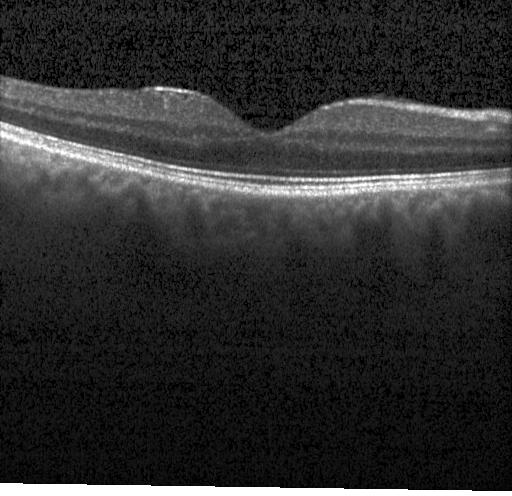
Assessment: no choroidal neovascularization, diabetic macular edema, or drusen.